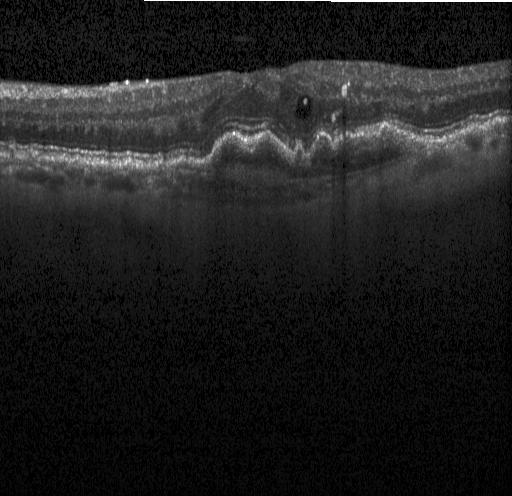

OCT B-scan, Heidelberg Spectralis OCT system. Assessment: a choroidal neovascular membrane.